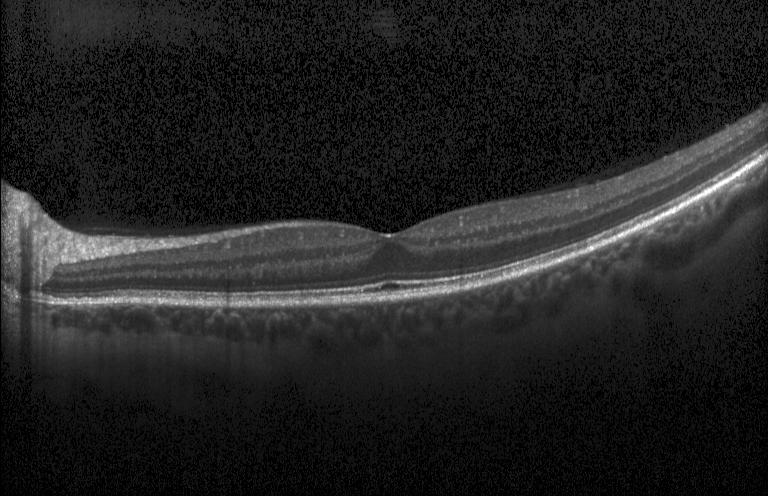

This B-scan demonstrates no choroidal neovascularization, no diabetic macular edema, and no drusen.